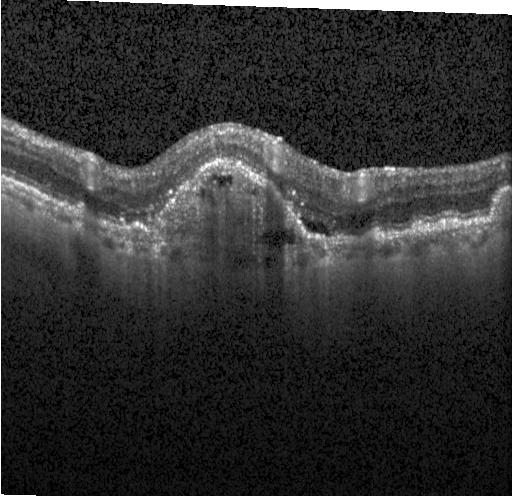
Heidelberg Spectralis OCT system. Through the macula. Retinal OCT cross-section
This B-scan demonstrates a choroidal neovascular membrane.